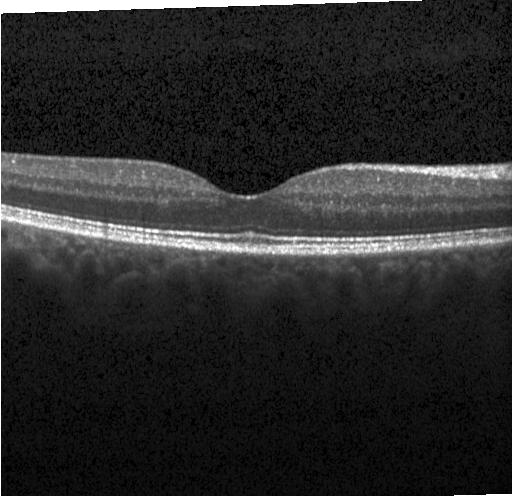
Diagnosis: neither choroidal neovascularization, diabetic macular edema, nor drusen.